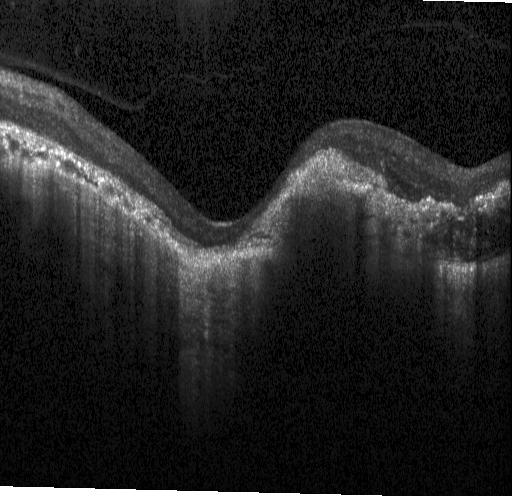

Heidelberg Spectralis. OCT B-scan
Finding: choroidal neovascularization.